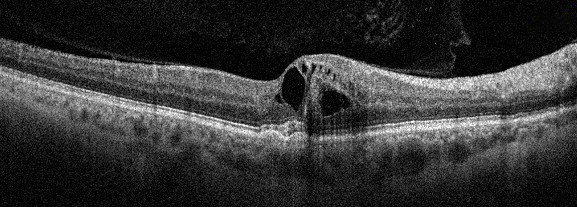
OCT line scan · acquired on an Optovue Avanti RTVue XR · fovea-centered — Diagnosis: retinal vein occlusion (RVO).